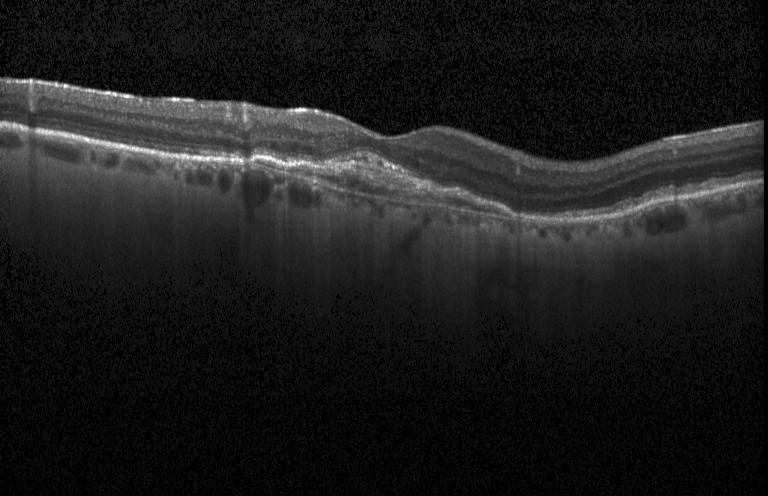

Finding: CNV.